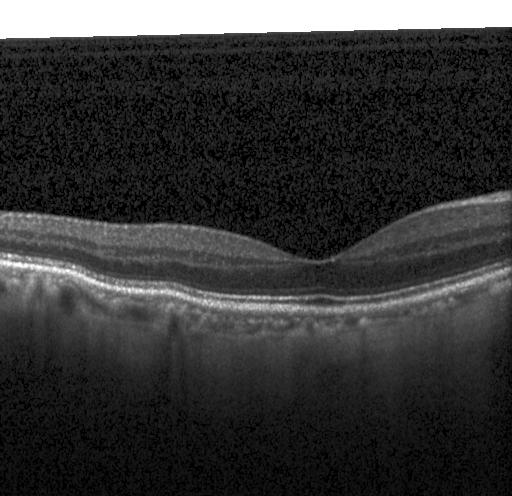
OCT scan showing no evidence of choroidal neovascularization, diabetic macular edema, or drusen.